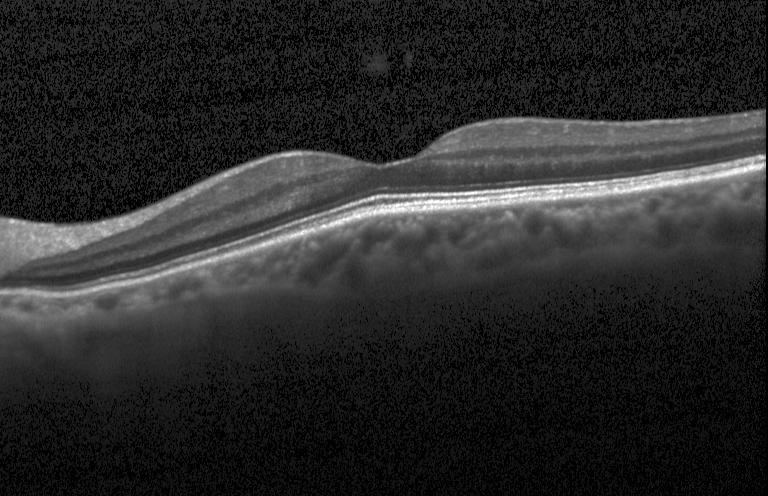

Fovea-centered, Heidelberg Spectralis, OCT line scan — No evidence of choroidal neovascularization, diabetic macular edema, or drusen.